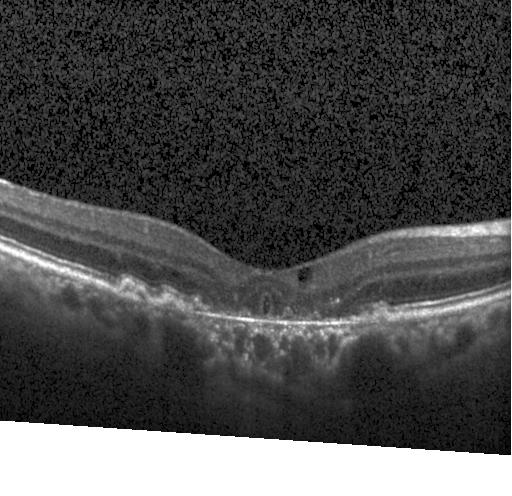
The scan shows choroidal neovascularization.